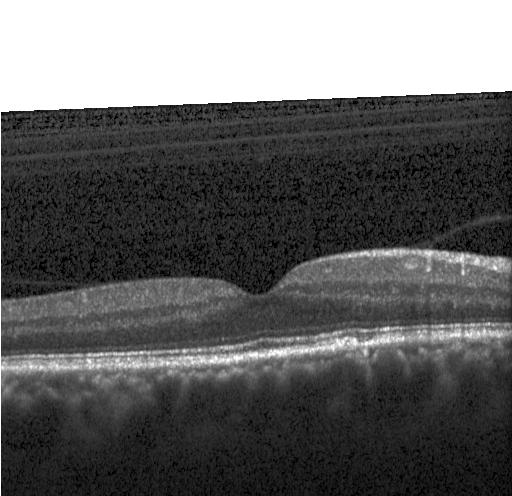 Instrument: Heidelberg Spectralis · spectral-domain OCT · retinal OCT B-scan
Finding: no choroidal neovascularization, diabetic macular edema, or drusen.